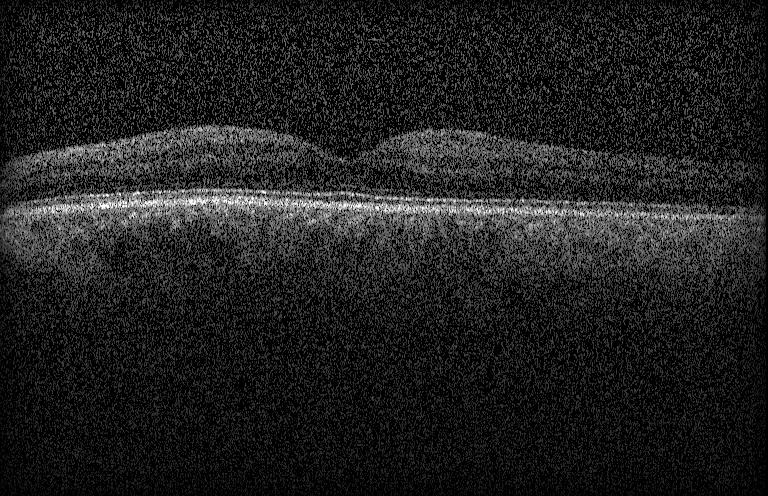
Impression: no choroidal neovascularization, diabetic macular edema, or drusen.